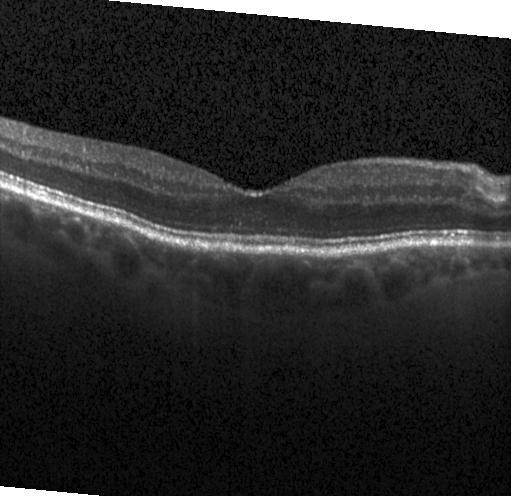

Assessment: no choroidal neovascularization, no diabetic macular edema, and no drusen.